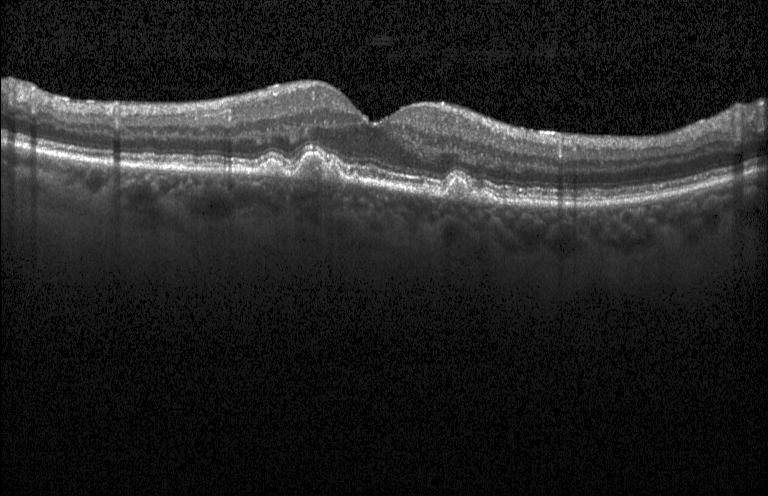 OCT B-scan.
Diagnosis: sub-RPE drusenoid deposits.